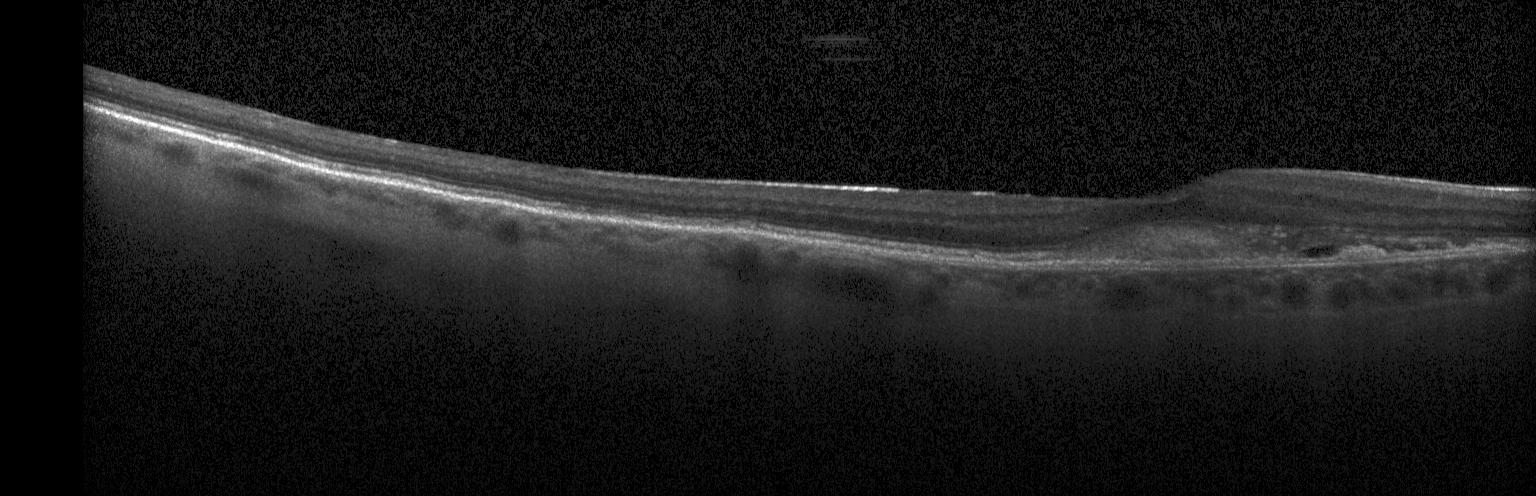
OCT scan showing a choroidal neovascular membrane.